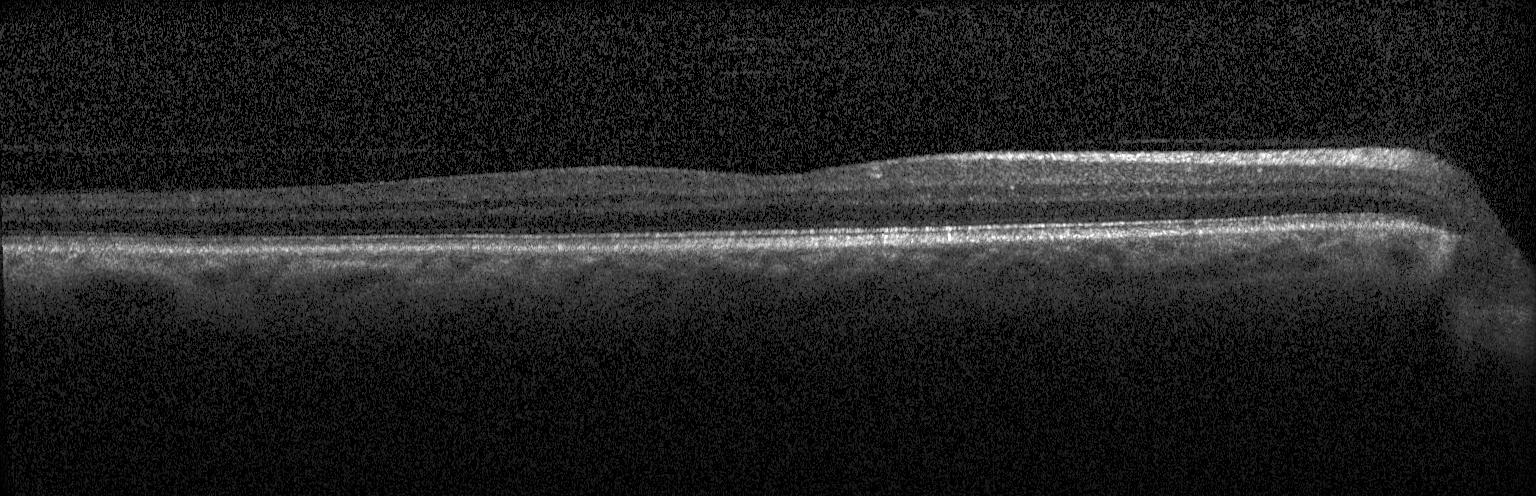

OCT B-scan.
Impression: no choroidal neovascularization, no diabetic macular edema, and no drusen.